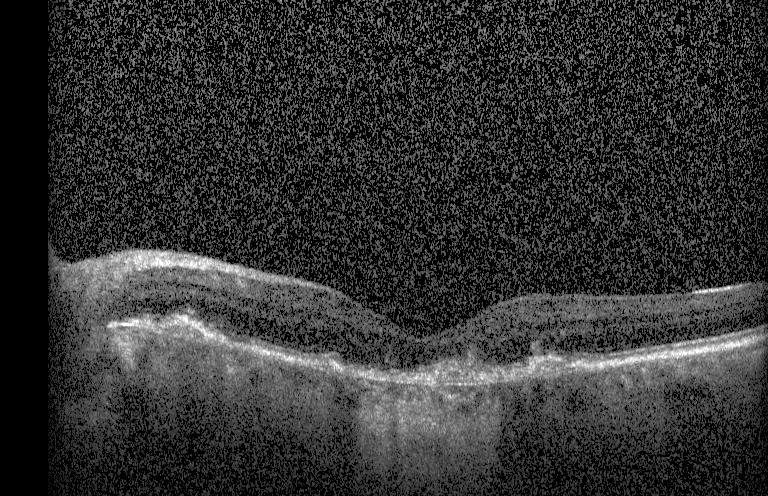

OCT line scan
Finding: CNV.